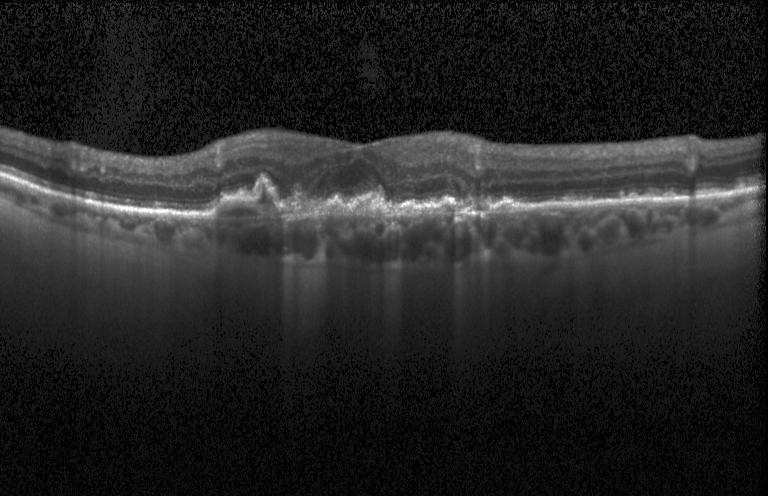
OCT line scan; SD-OCT; fovea-centered; acquired on a Heidelberg Spectralis.
Macular OCT: a choroidal neovascular membrane.